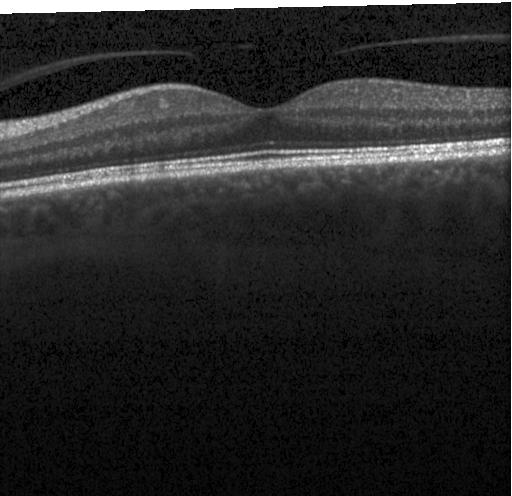

Heidelberg Spectralis; macular scan; optical coherence tomography B-scan; spectral-domain OCT.
Impression: no choroidal neovascularization, no diabetic macular edema, and no drusen.